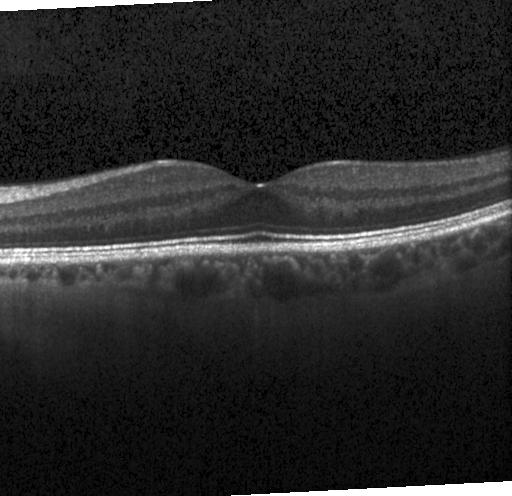

Diagnosis: no choroidal neovascularization, no diabetic macular edema, and no drusen.